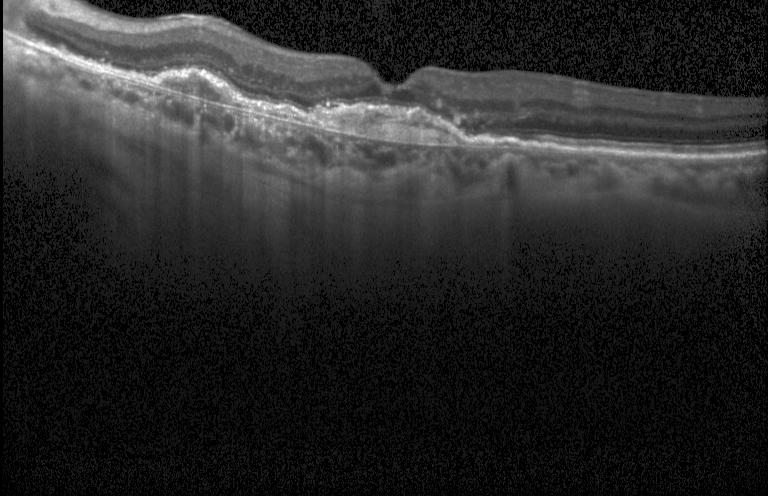 Assessment: a choroidal neovascular membrane.